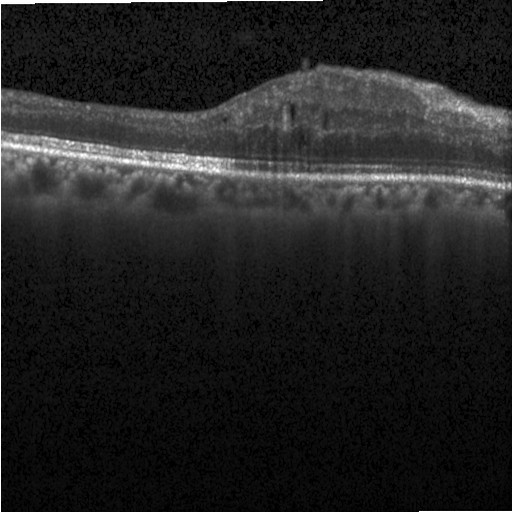

SD-OCT, retinal OCT B-scan, centered on the fovea
Finding: diabetic macular edema.